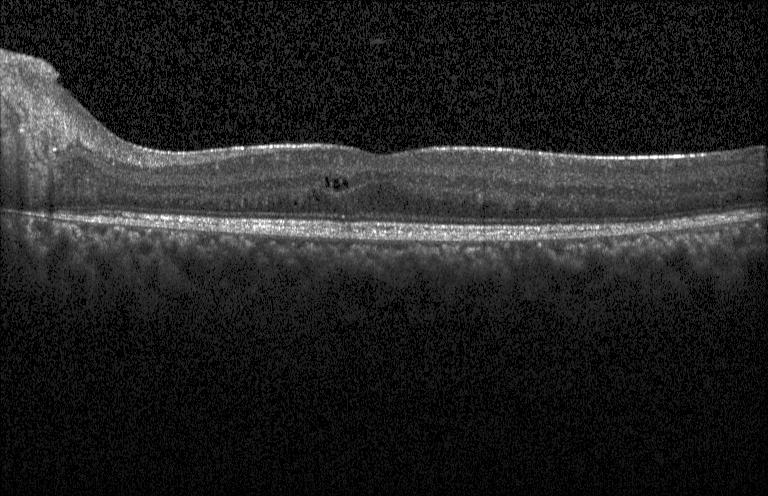 Fovea-centered · spectral-domain optical coherence tomography · OCT line scan · Heidelberg Spectralis
Finding: DME.